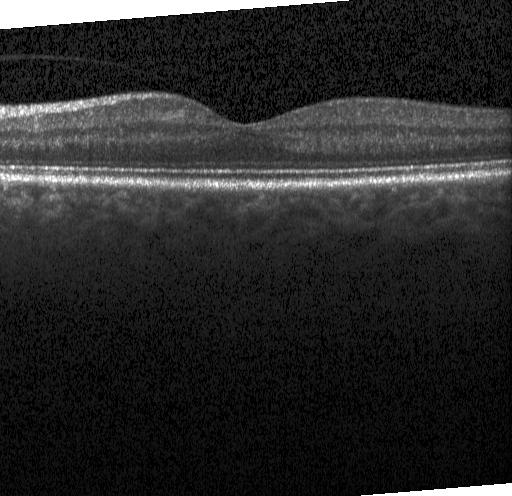 Diagnosis: no CNV, DME, or drusen.